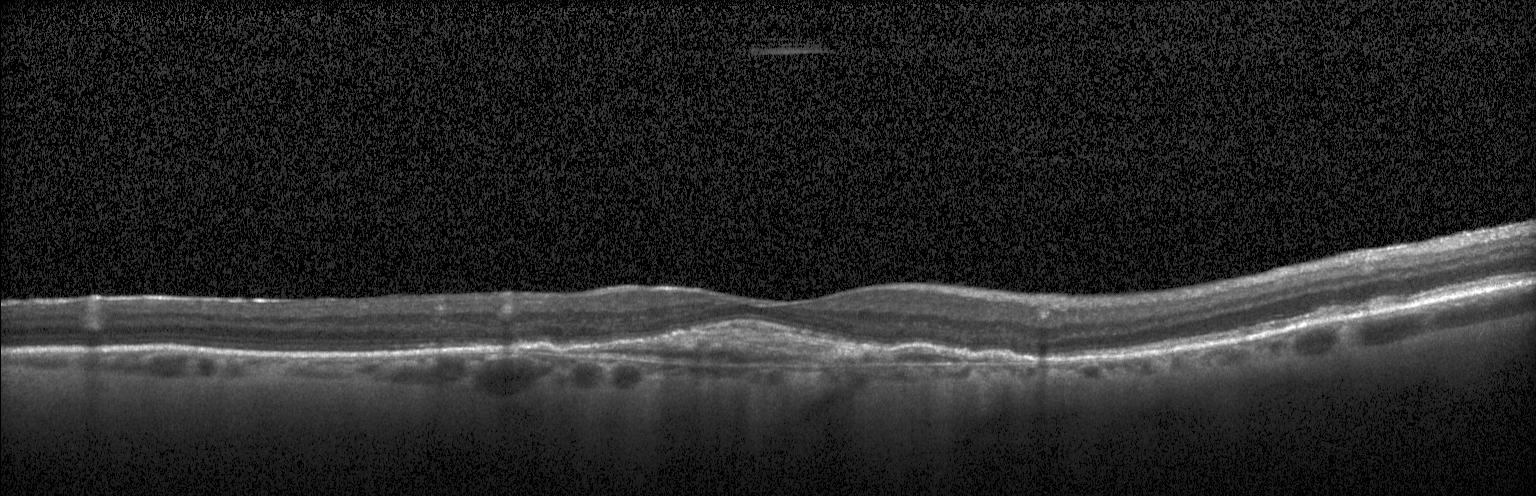

Spectral-domain OCT B-scan: a choroidal neovascular membrane.